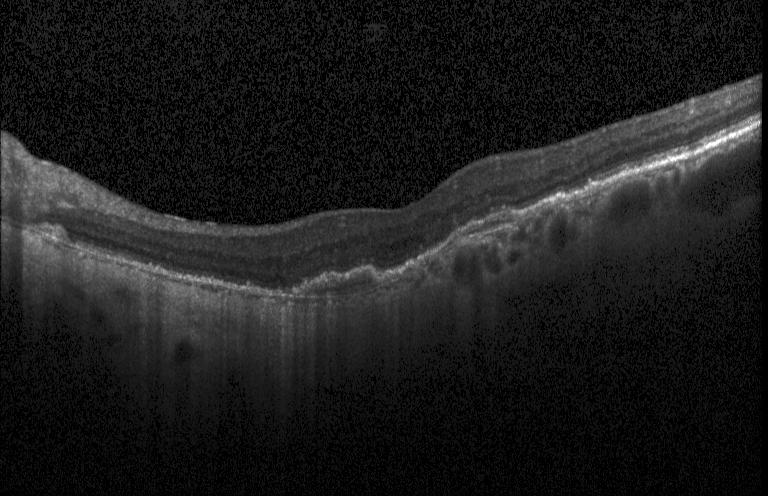

Macular OCT: choroidal neovascularization (CNV).